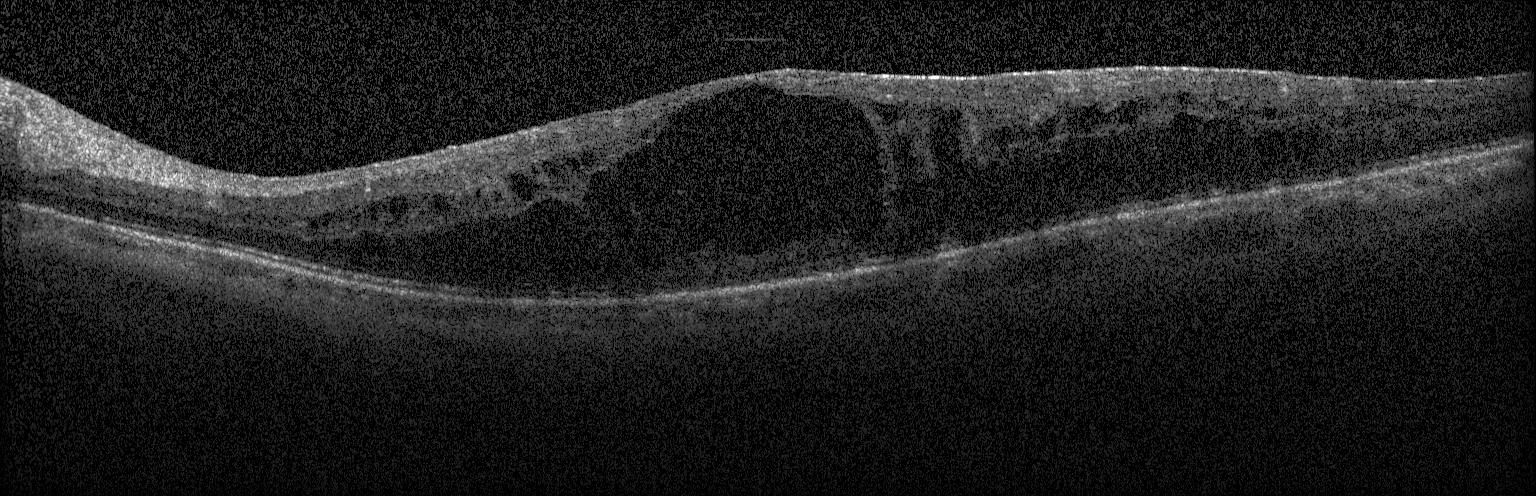
OCT B-scan
Diagnosis: diabetic macular edema.